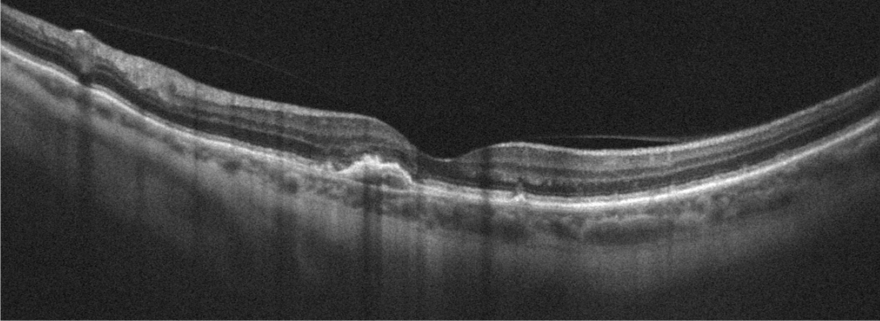 OCT line scan. Dx: AMD.